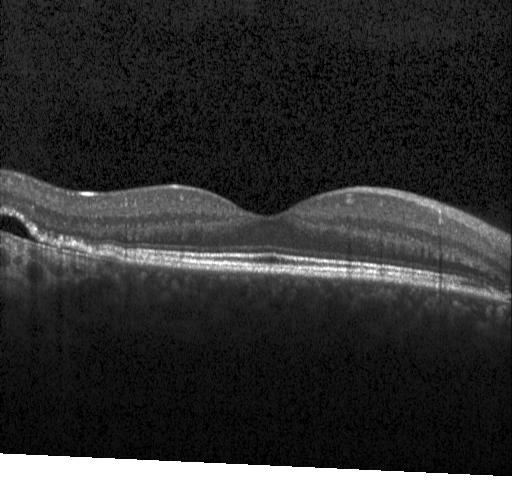

Dx: choroidal neovascularization.